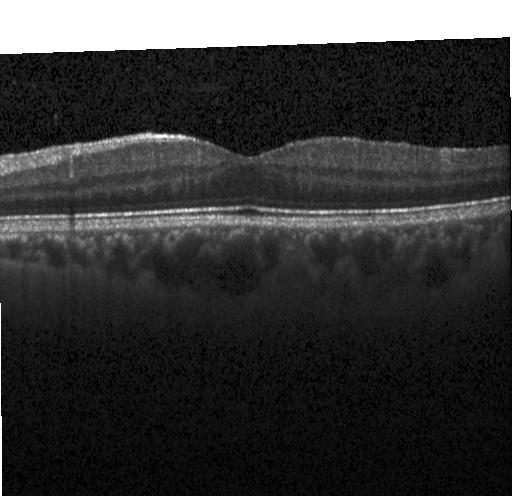 OCT B-scan — The scan shows no choroidal neovascularization, no diabetic macular edema, and no drusen.